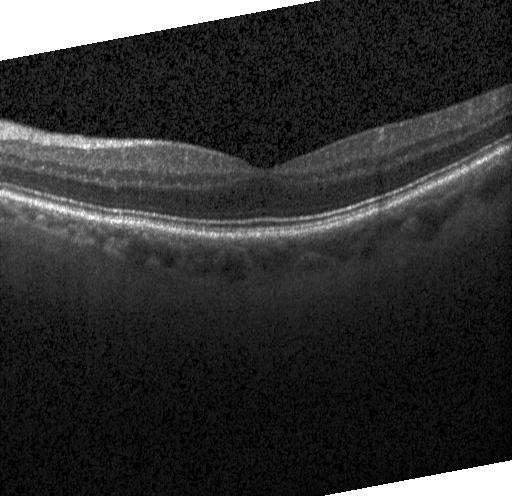 Spectral-domain OCT B-scan: no choroidal neovascularization, no diabetic macular edema, and no drusen.